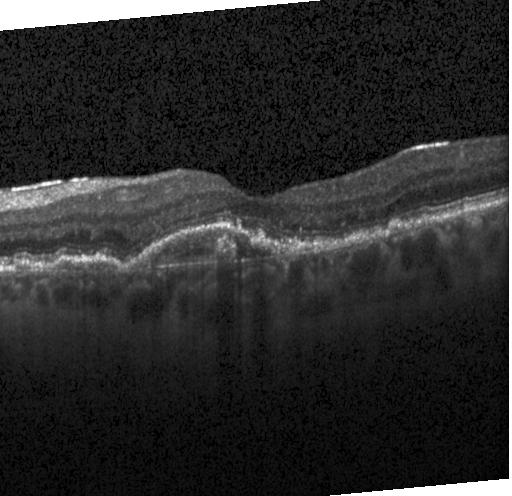
SD-OCT. Heidelberg Spectralis OCT system. Optical coherence tomography scan. Horizontal scan through the fovea
Dx: choroidal neovascularization.